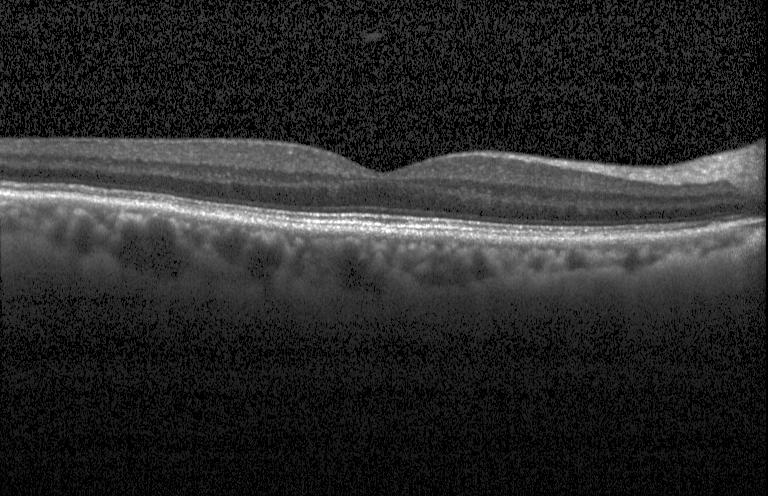 OCT B-scan.
Diagnosis: no evidence of CNV, DME, or drusen.